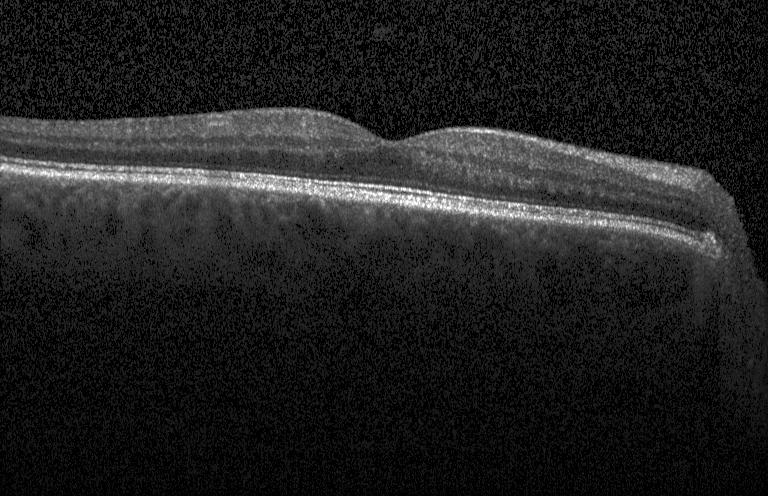
Retinal OCT cross-section.
This B-scan demonstrates neither choroidal neovascularization, diabetic macular edema, nor drusen.